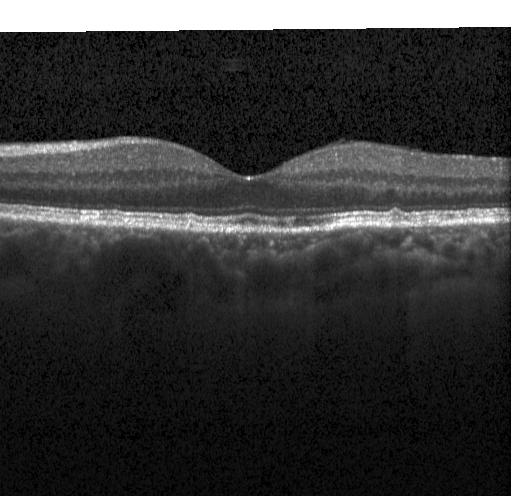 OCT line scan. Centered on the fovea.
Impression: drusen.